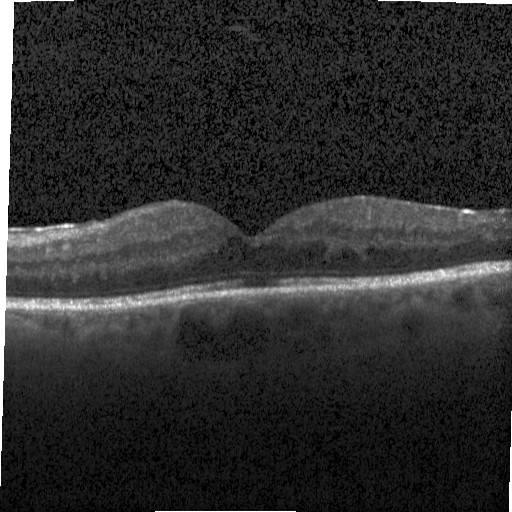

Horizontal scan through the fovea · spectral-domain OCT · retinal OCT B-scan
Finding: diabetic macular edema (DME).